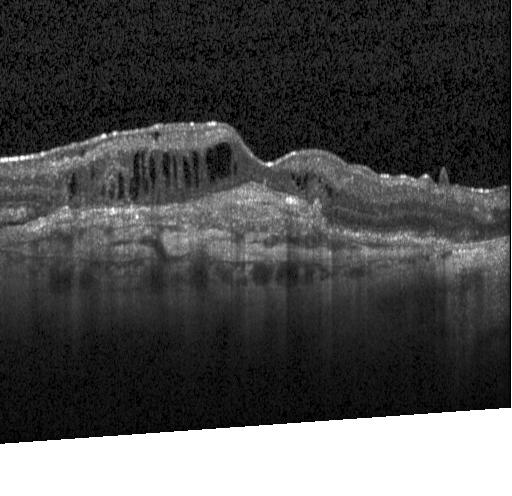

Dx: a choroidal neovascular membrane.